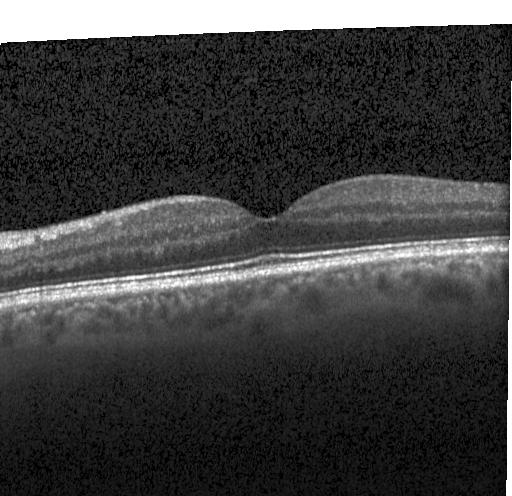

Retinal OCT cross-section. Impression: no CNV, no DME, and no drusen.